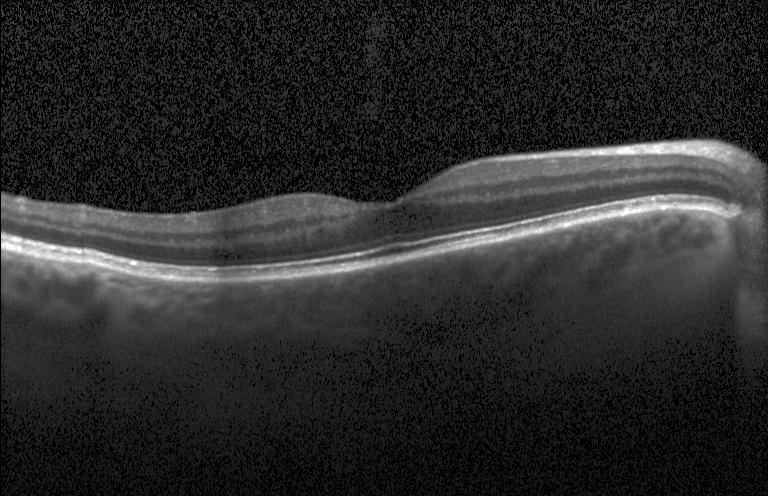 Macular OCT demonstrating no evidence of choroidal neovascularization, diabetic macular edema, or drusen.